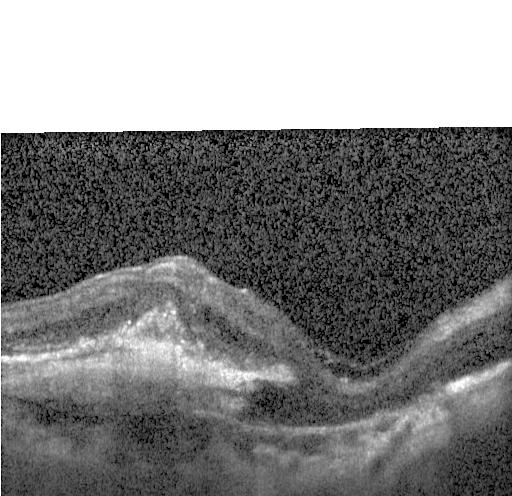 Macular OCT: CNV.